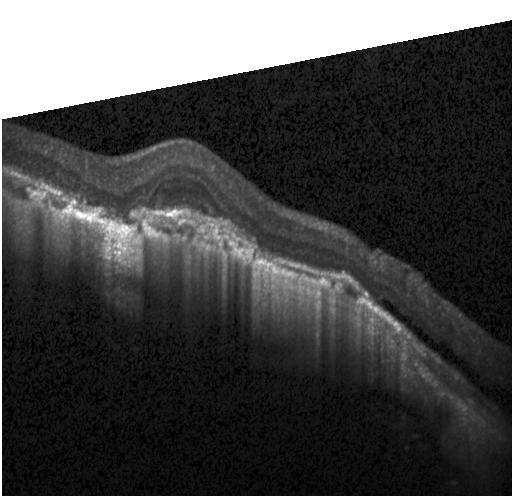

OCT B-scan showing a choroidal neovascular membrane.